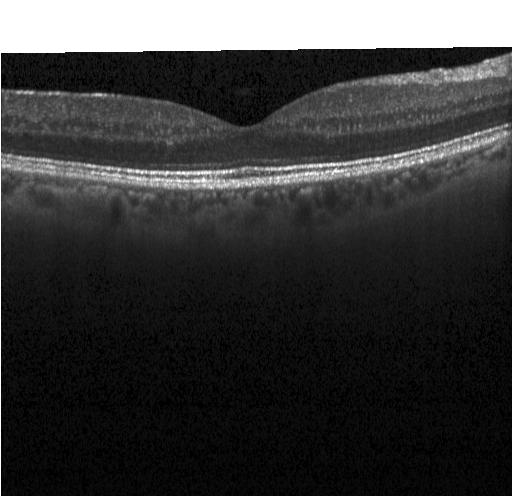 OCT line scan; Heidelberg Spectralis OCT system; spectral-domain optical coherence tomography; horizontal scan through the fovea. Impression: no evidence of choroidal neovascularization, diabetic macular edema, or drusen.